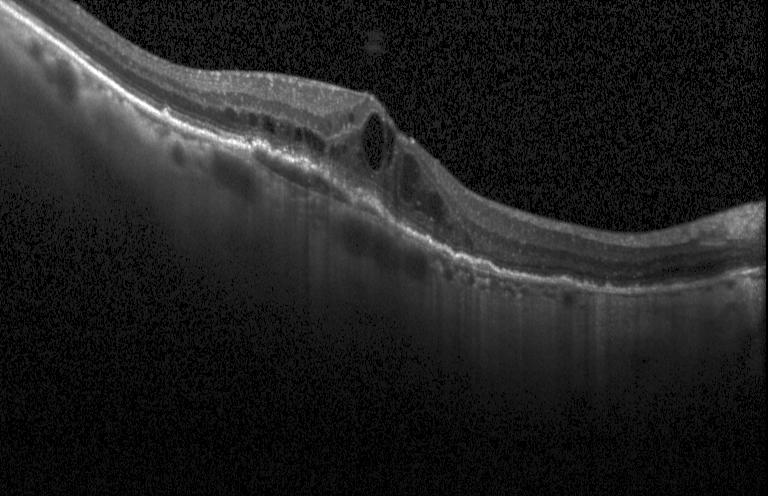

Optical coherence tomography scan · Heidelberg Spectralis OCT system · spectral-domain OCT. Impression: a choroidal neovascular membrane.